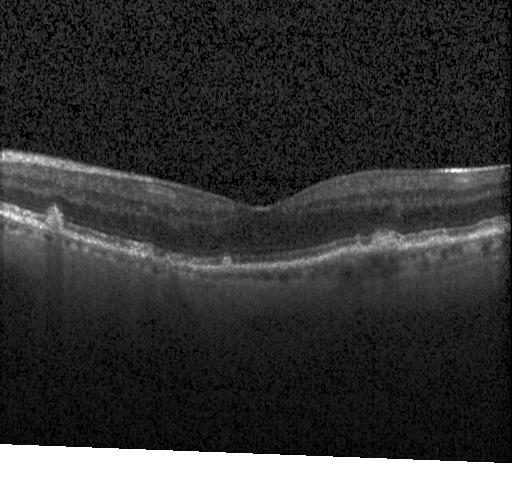 Macular OCT: drusen.